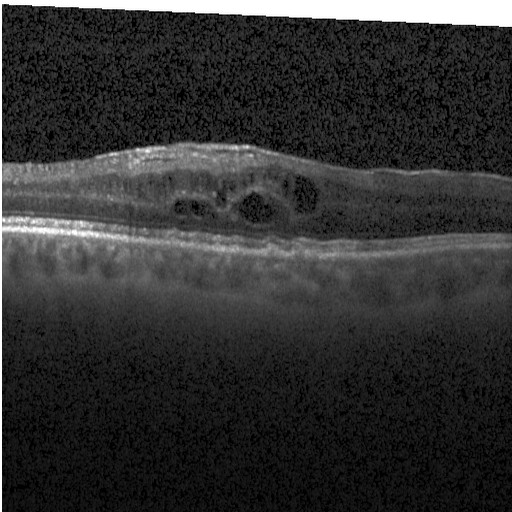 Finding: DME.